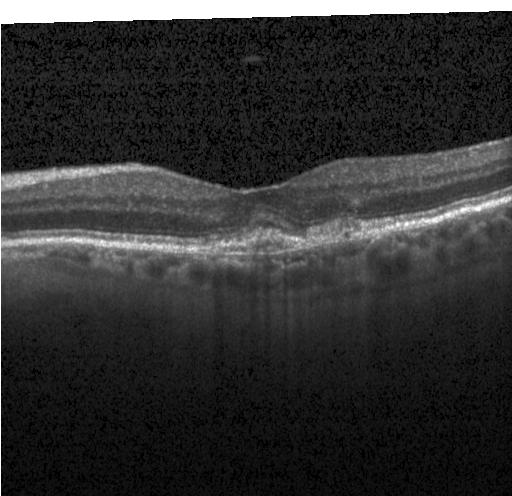

Impression: choroidal neovascularization (CNV).